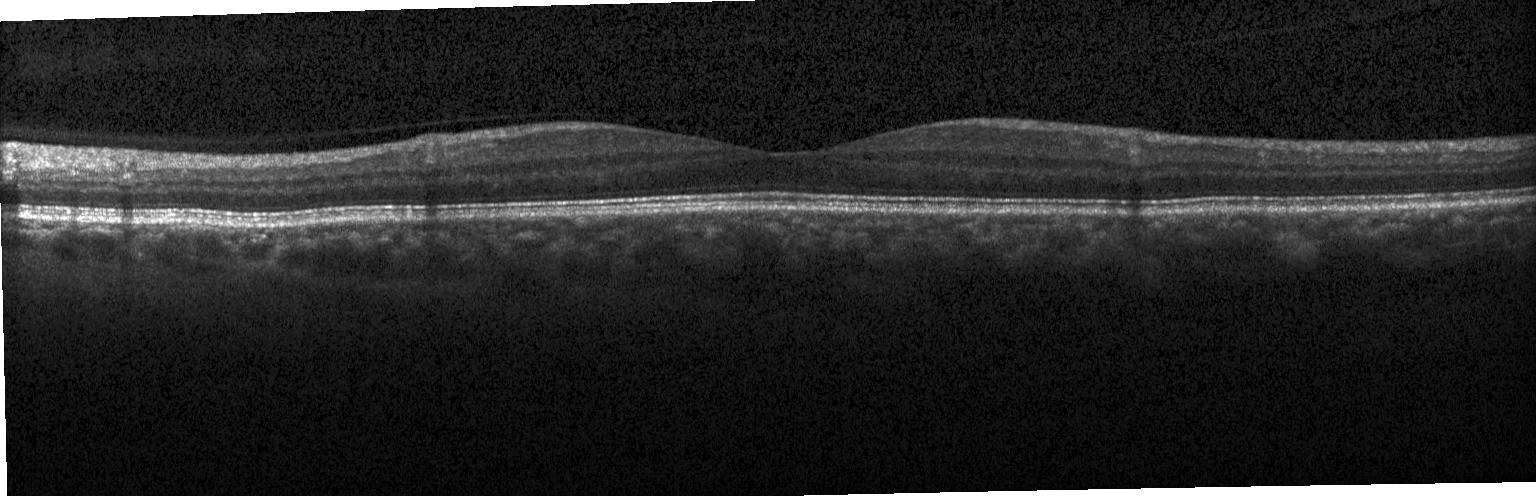
Optical coherence tomography scan; horizontal scan through the fovea; acquired on a Heidelberg Spectralis
No CNV, no DME, and no drusen.